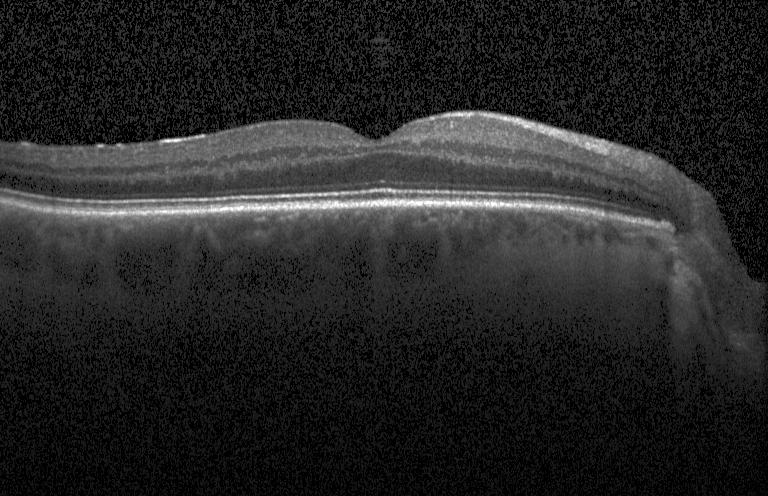

Macular OCT: no evidence of choroidal neovascularization, diabetic macular edema, or drusen.